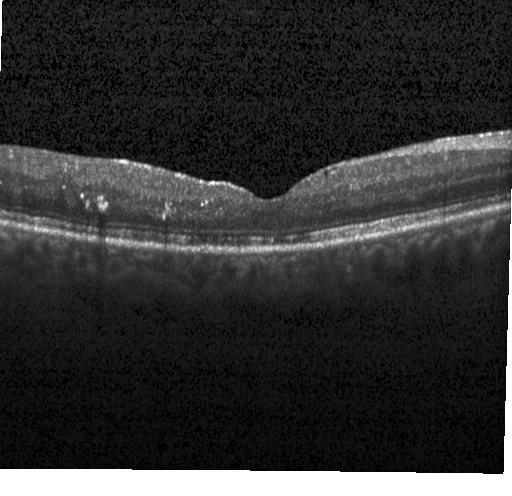

Finding: DME.